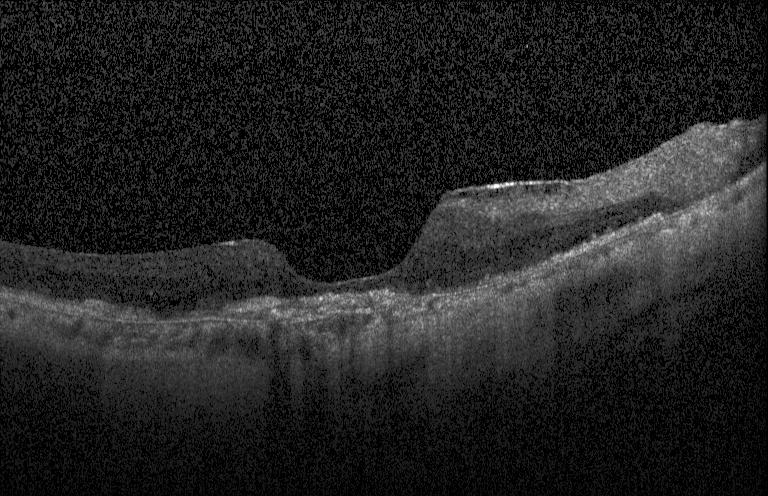

OCT B-scan. Impression: a choroidal neovascular membrane.